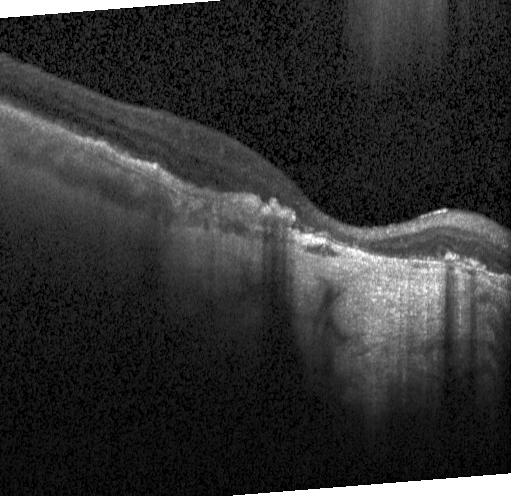
Through the macula · Heidelberg Spectralis · retinal OCT B-scan · SD-OCT.
Macular OCT: choroidal neovascularization (CNV).